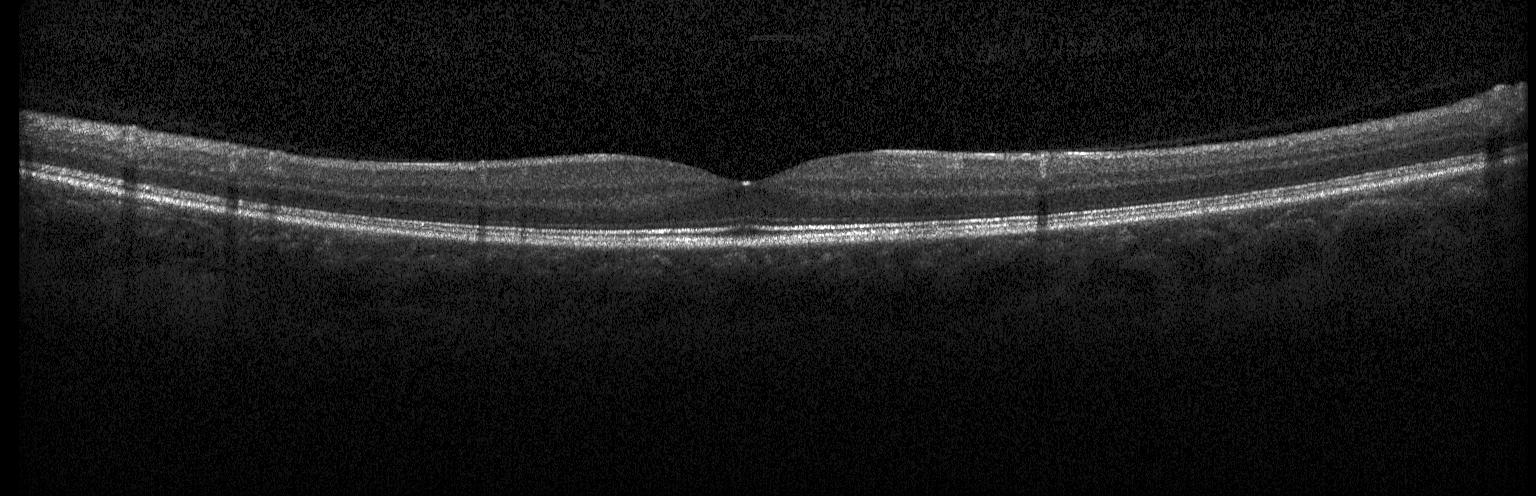 Retinal OCT B-scan, instrument: Heidelberg Spectralis, spectral-domain optical coherence tomography — Finding: no choroidal neovascularization, diabetic macular edema, or drusen.